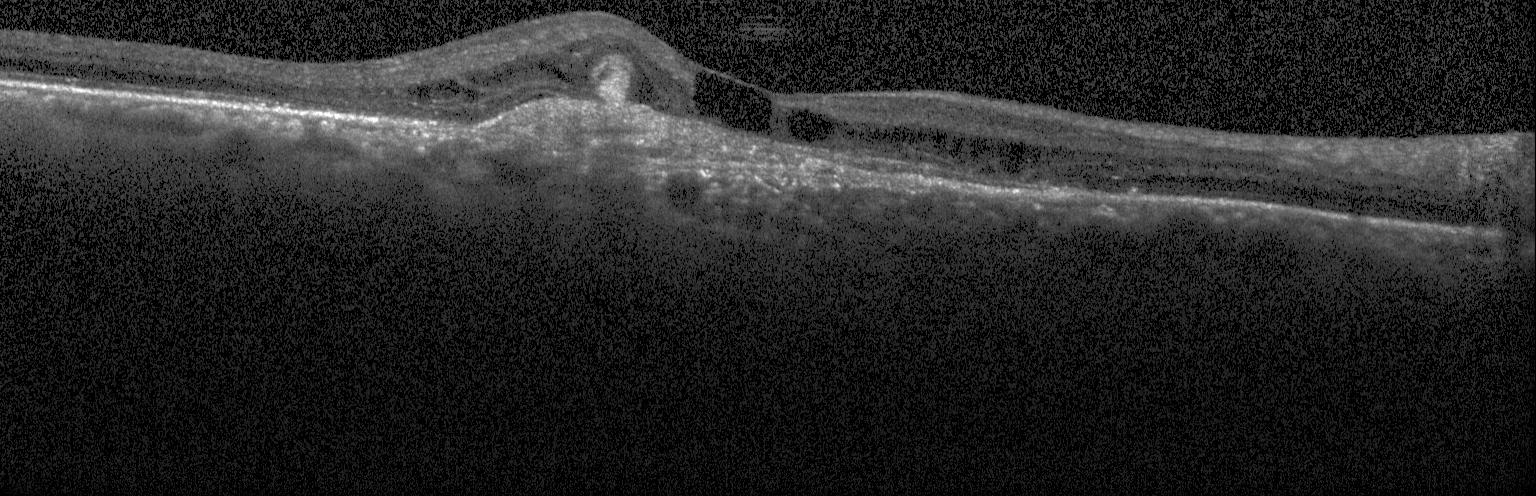
Spectral-domain OCT B-scan: a choroidal neovascular membrane.